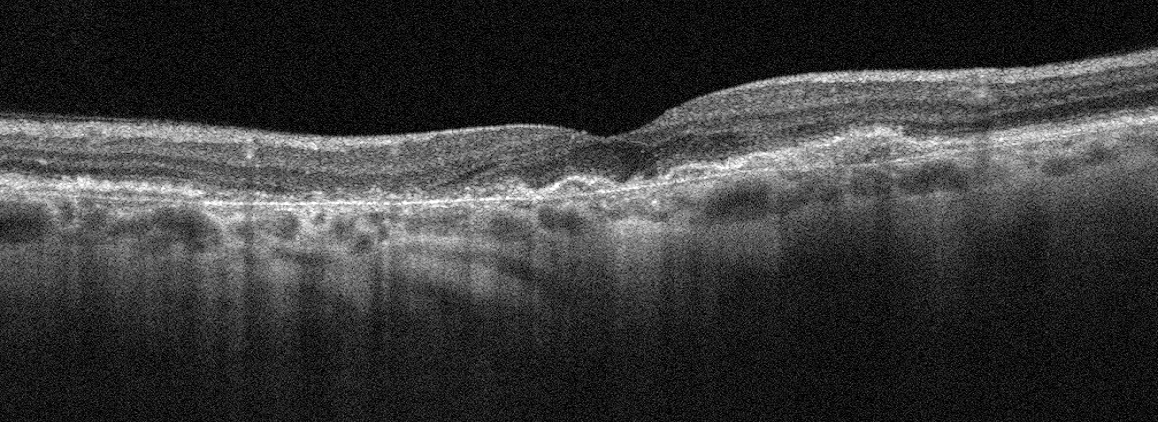 OS. OCT B-scan
Dx: age-related macular degeneration.